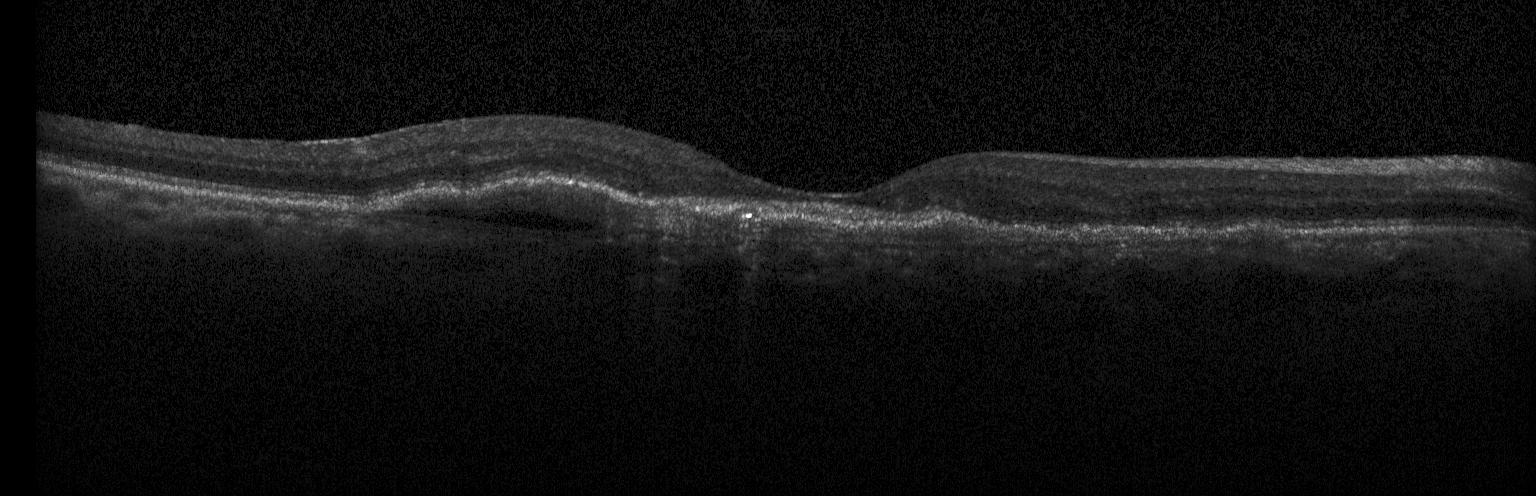 Assessment: CNV.